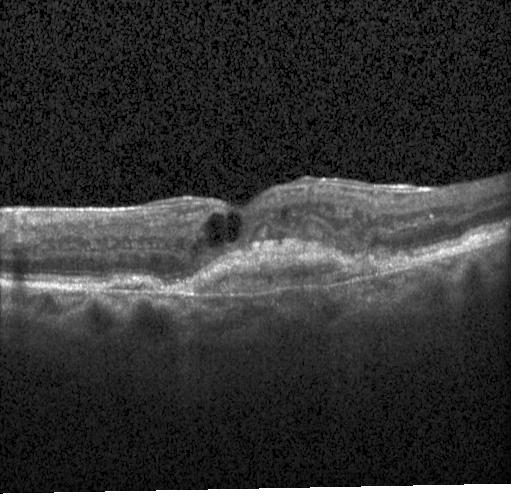
Assessment: a choroidal neovascular membrane.